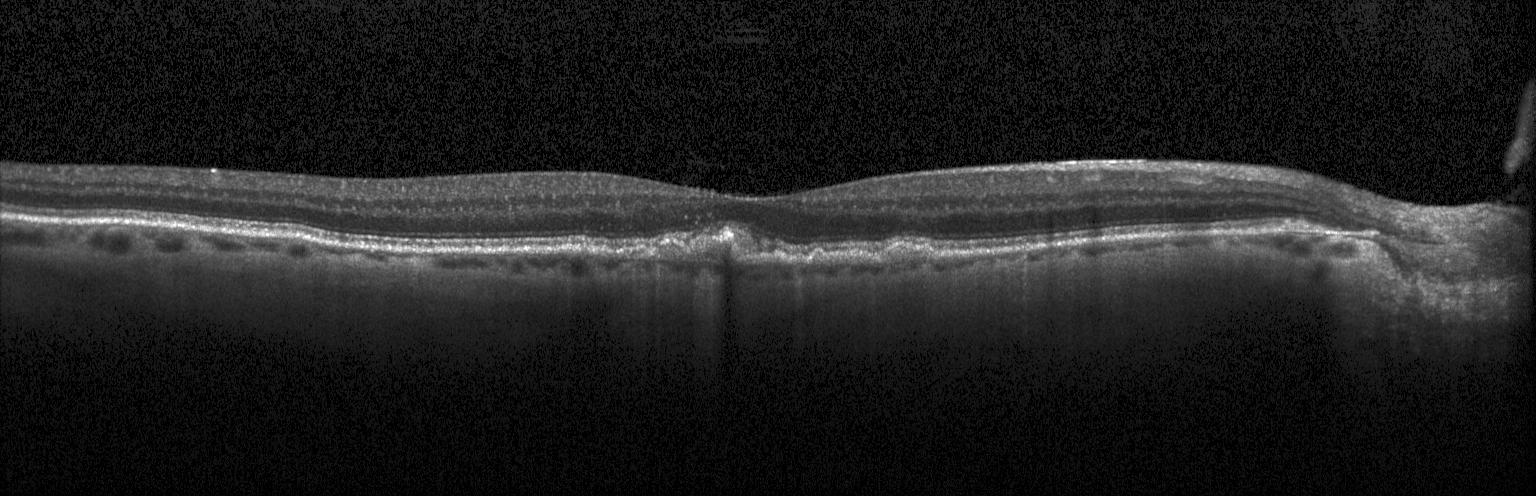

Retinal OCT cross-section, instrument: Heidelberg Spectralis, SD-OCT, horizontal scan through the fovea.
Impression: multiple drusen.